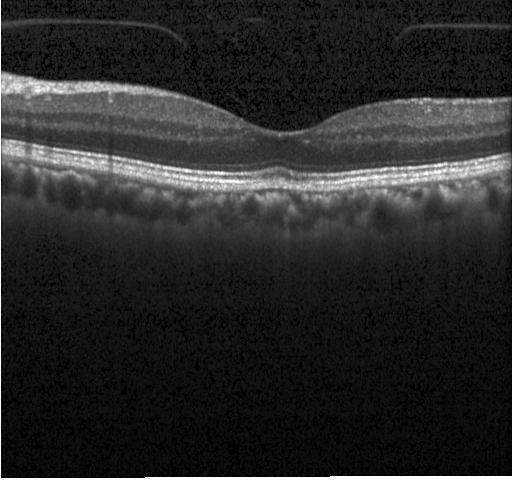 Spectral-domain OCT · retinal OCT cross-section.
OCT finding: no CNV, DME, or drusen.